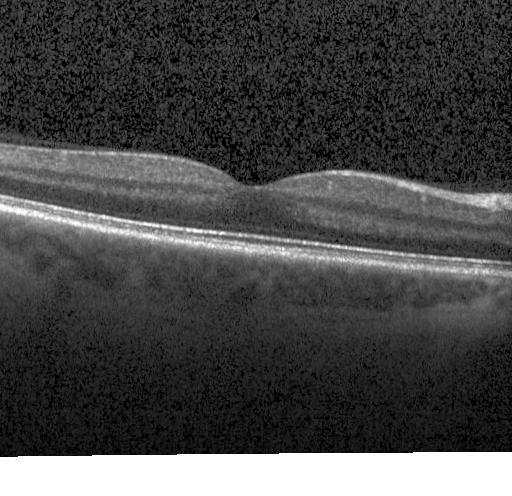

Heidelberg Spectralis · retinal OCT B-scan
This B-scan demonstrates no evidence of choroidal neovascularization, diabetic macular edema, or drusen.